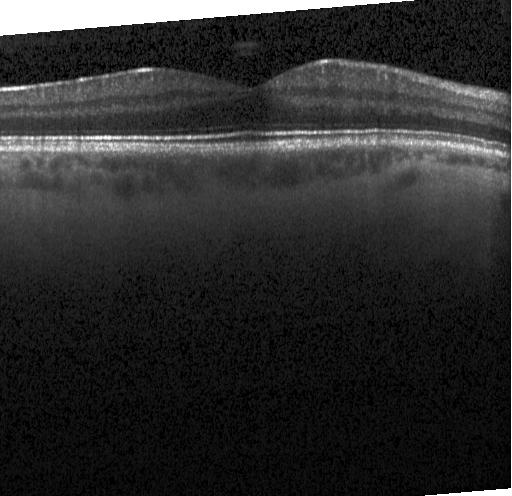

Through the macula; spectral-domain OCT; OCT line scan; acquired on a Heidelberg Spectralis.
Diagnosis: neither choroidal neovascularization, diabetic macular edema, nor drusen.